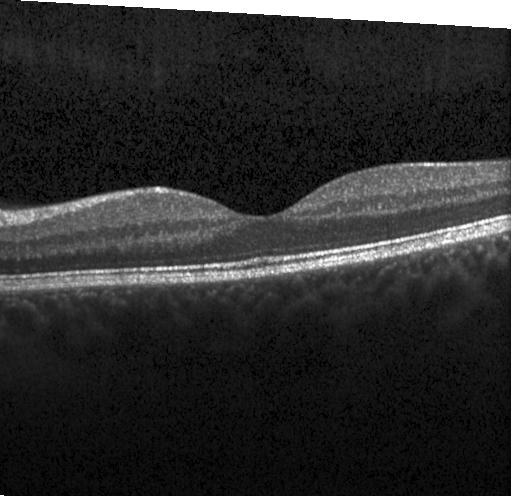

Retinal OCT cross-section
The scan shows no evidence of choroidal neovascularization, diabetic macular edema, or drusen.